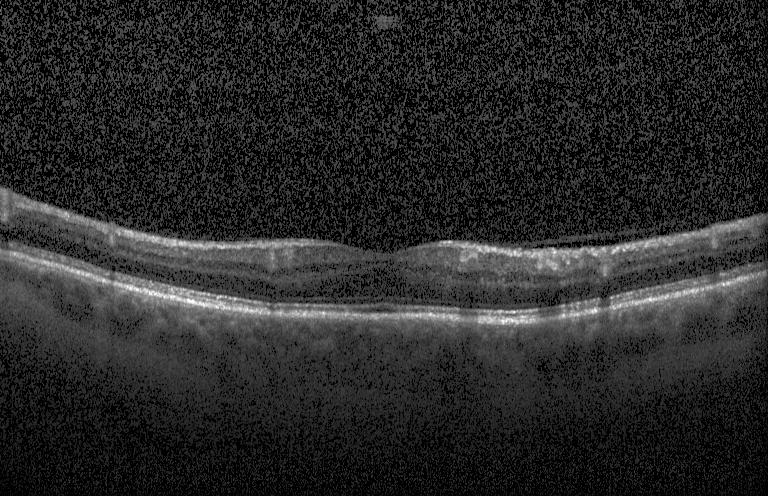
Finding: no choroidal neovascularization, no diabetic macular edema, and no drusen.